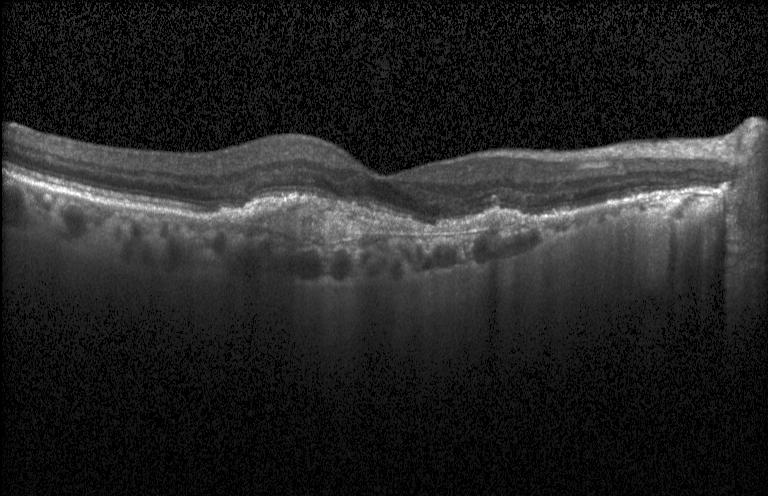 Impression: choroidal neovascularization (CNV).